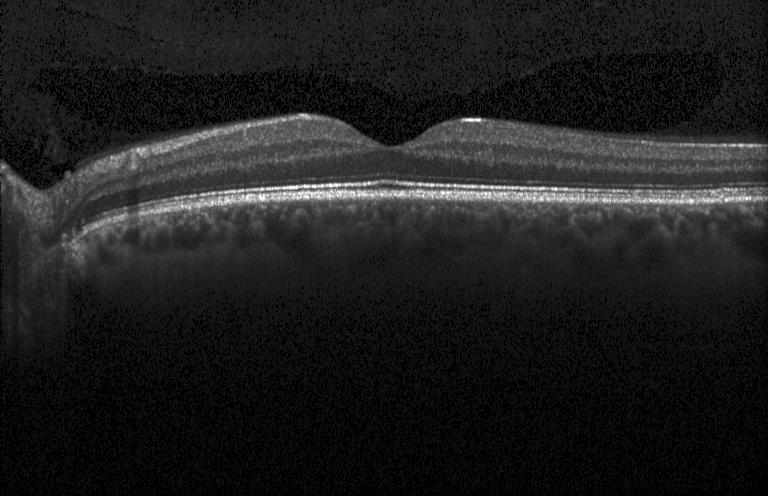 Impression: neither choroidal neovascularization, diabetic macular edema, nor drusen.